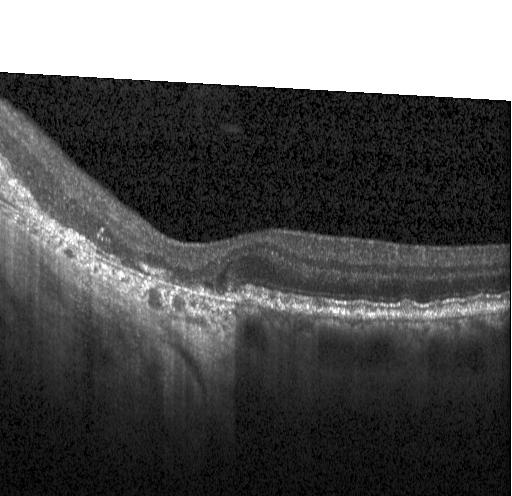 OCT finding: a choroidal neovascular membrane.